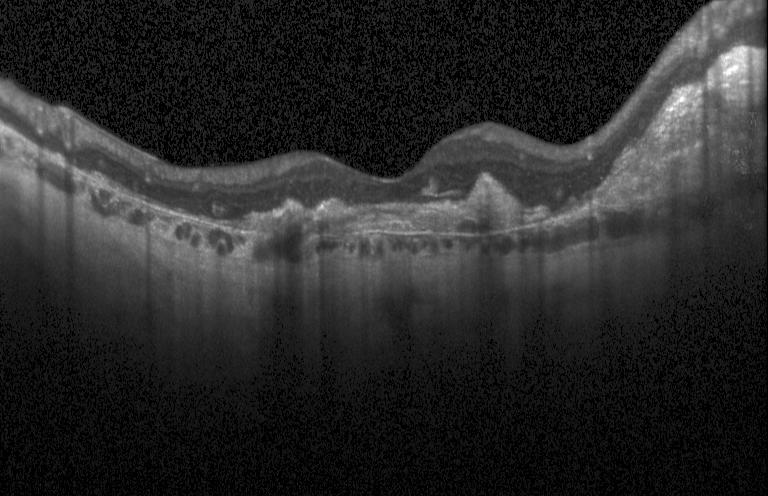 OCT B-scan showing choroidal neovascularization (CNV).